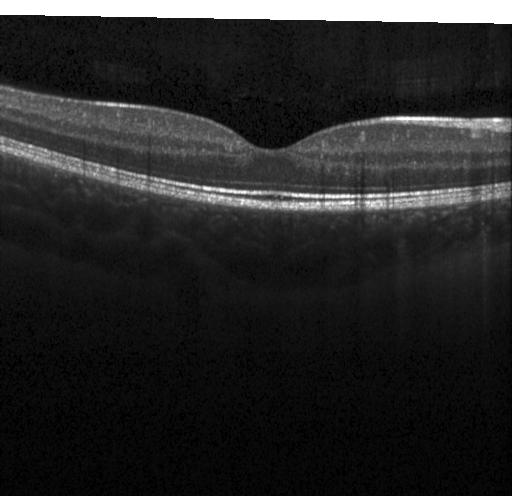
Optical coherence tomography scan. Impression: neither CNV, DME, nor drusen.